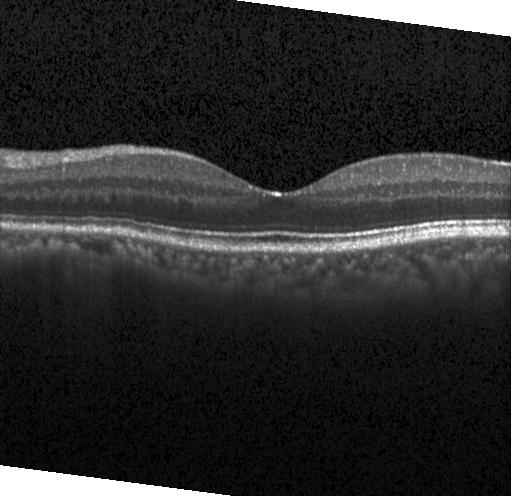
Instrument: Heidelberg Spectralis, through the macula, retinal OCT B-scan.
No CNV, no DME, and no drusen.